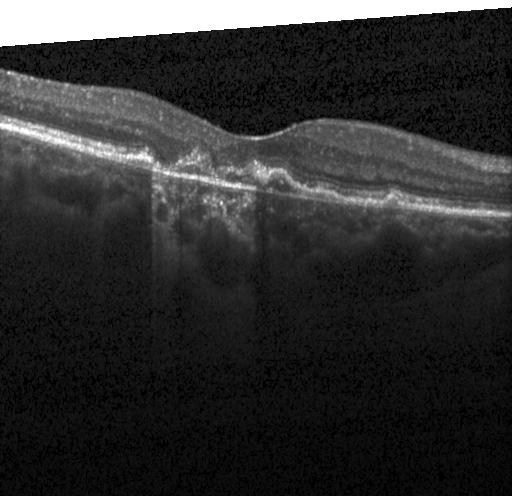 Diagnosis: choroidal neovascularization.